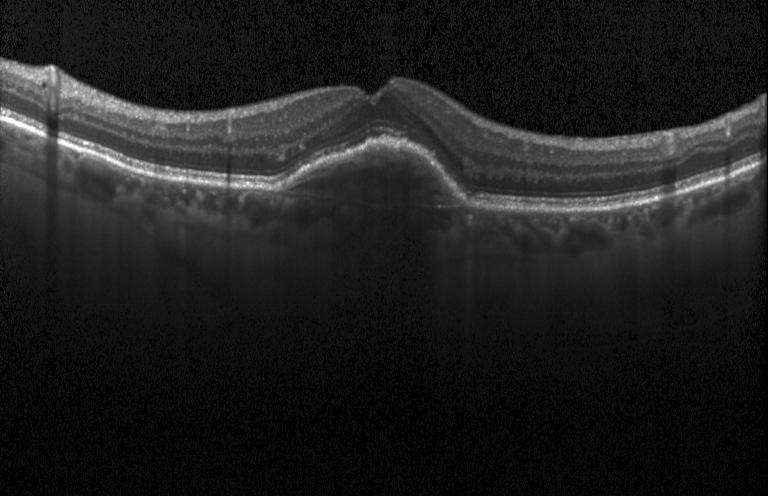
Diagnosis: a choroidal neovascular membrane.